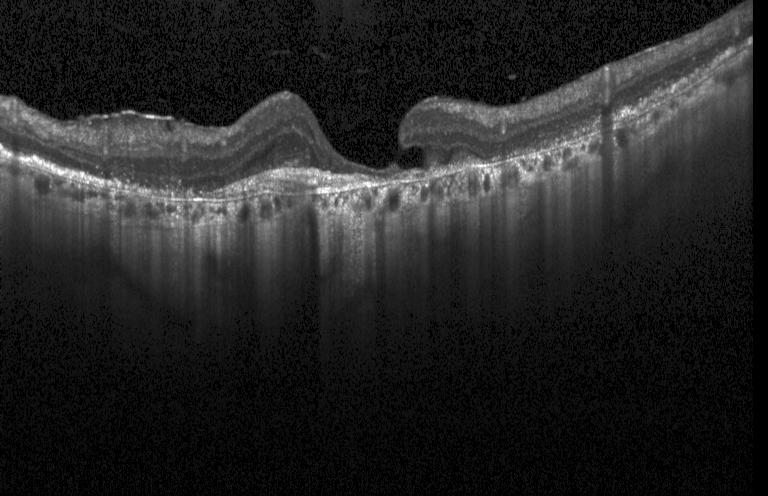
Macular scan · acquired on a Heidelberg Spectralis · OCT line scan · spectral-domain OCT.
Finding: a choroidal neovascular membrane.